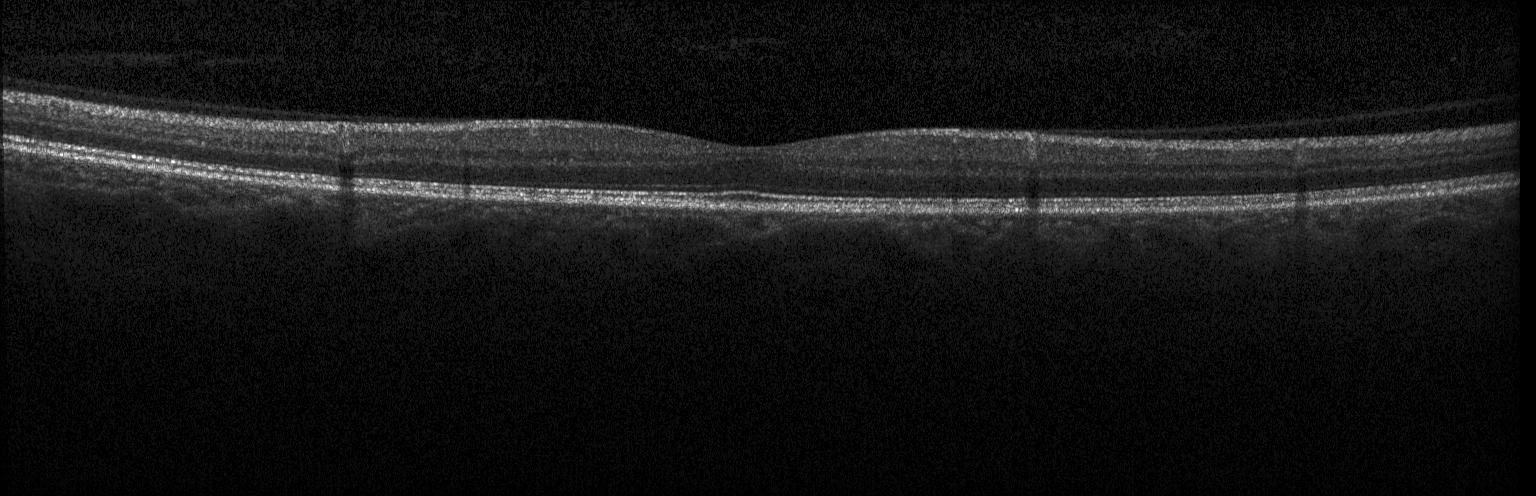

Macular scan. Retinal OCT cross-section. SD-OCT. Heidelberg Spectralis — The scan shows no choroidal neovascularization, diabetic macular edema, or drusen.